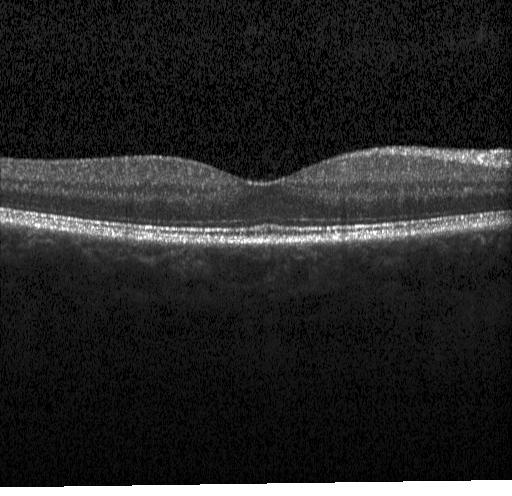 Heidelberg Spectralis OCT system. Centered on the fovea. Retinal OCT cross-section. Spectral-domain optical coherence tomography — Impression: no choroidal neovascularization, diabetic macular edema, or drusen.